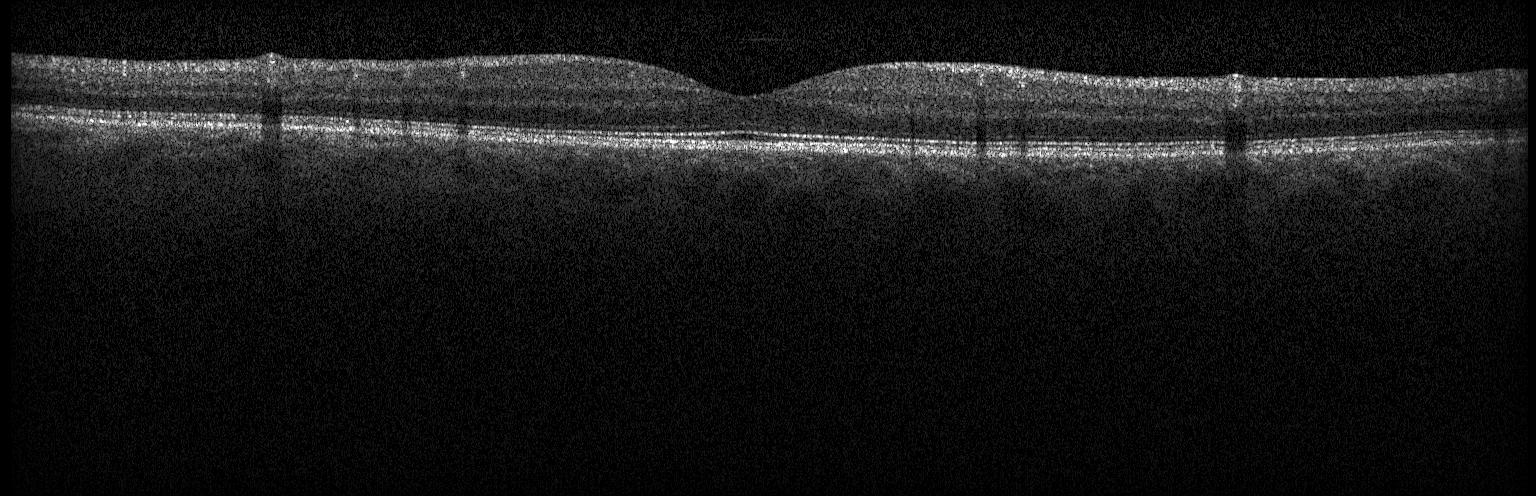

OCT B-scan — The scan shows neither choroidal neovascularization, diabetic macular edema, nor drusen.